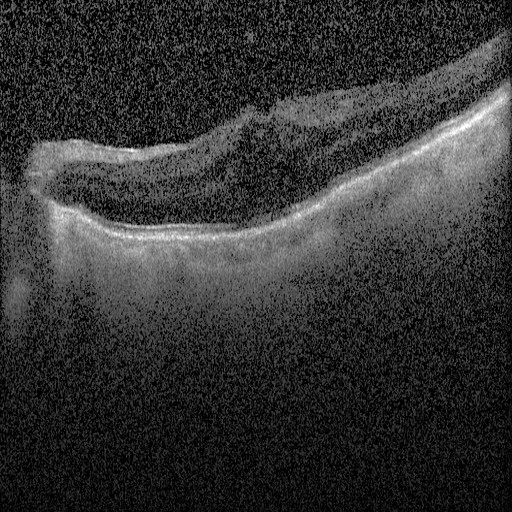

Retinal OCT B-scan
OCT finding: DME.